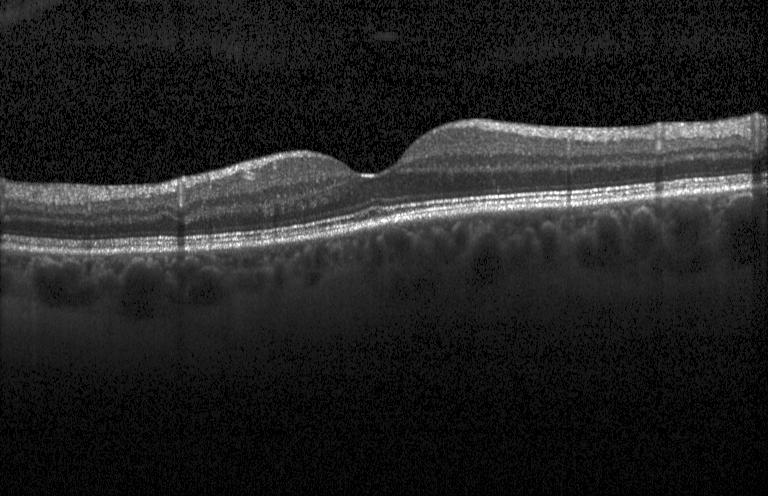

OCT line scan. SD-OCT.
Assessment: neither CNV, DME, nor drusen.